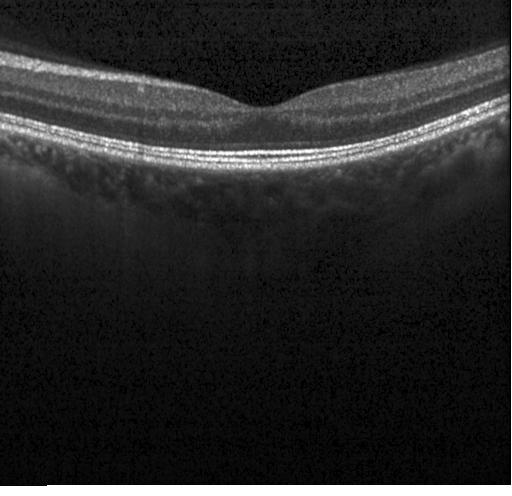

Optical coherence tomography scan — Dx: no choroidal neovascularization, diabetic macular edema, or drusen.